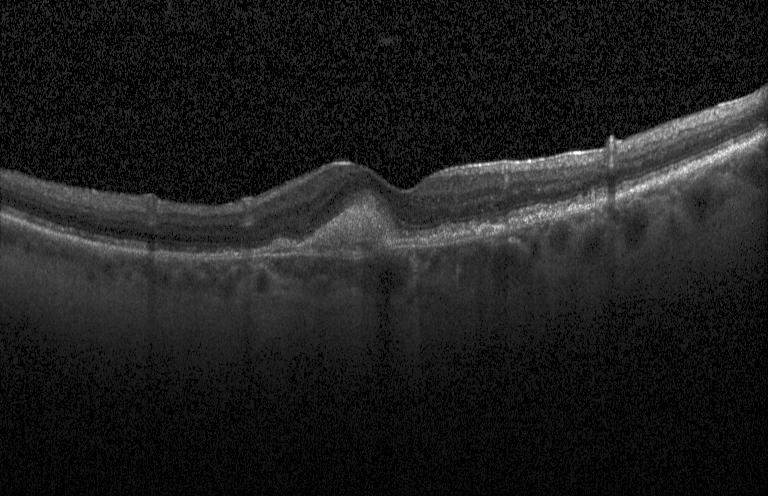
OCT line scan — CNV.